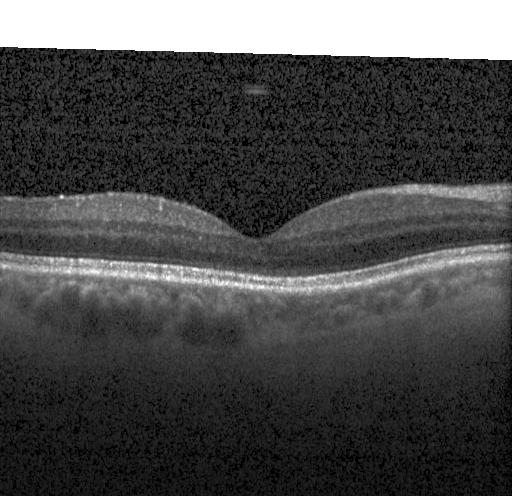 Heidelberg Spectralis. Optical coherence tomography scan
Impression: no CNV, no DME, and no drusen.